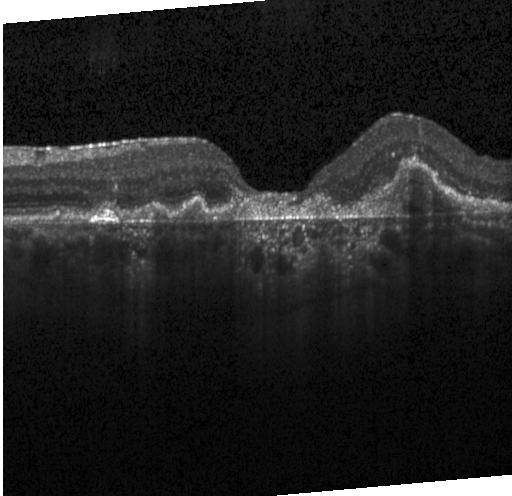 Fovea-centered. OCT line scan
Diagnosis: a choroidal neovascular membrane.